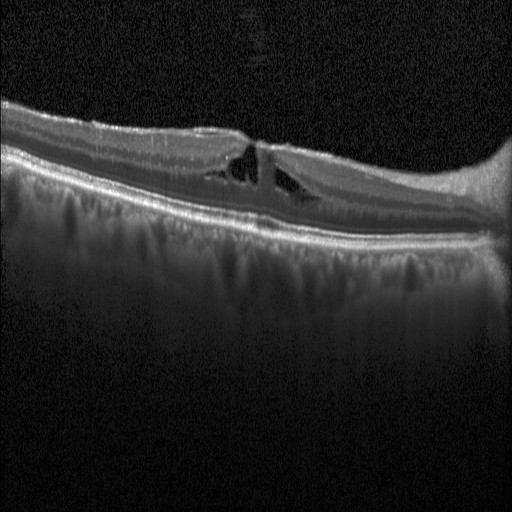

Through the macula · spectral-domain optical coherence tomography · retinal OCT cross-section — Finding: diabetic macular edema.